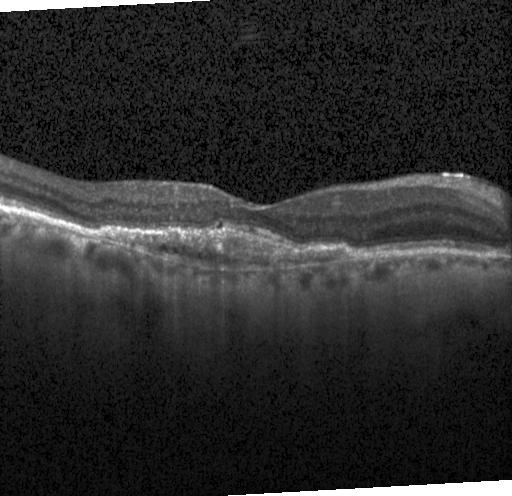

Spectral-domain OCT B-scan: a choroidal neovascular membrane.